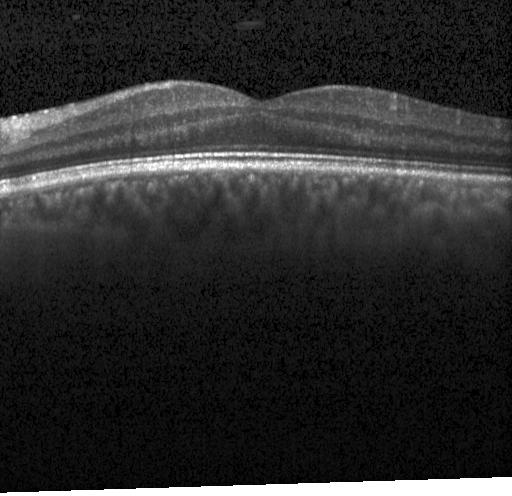 Spectral-domain OCT; retinal OCT cross-section. Impression: no CNV, DME, or drusen.